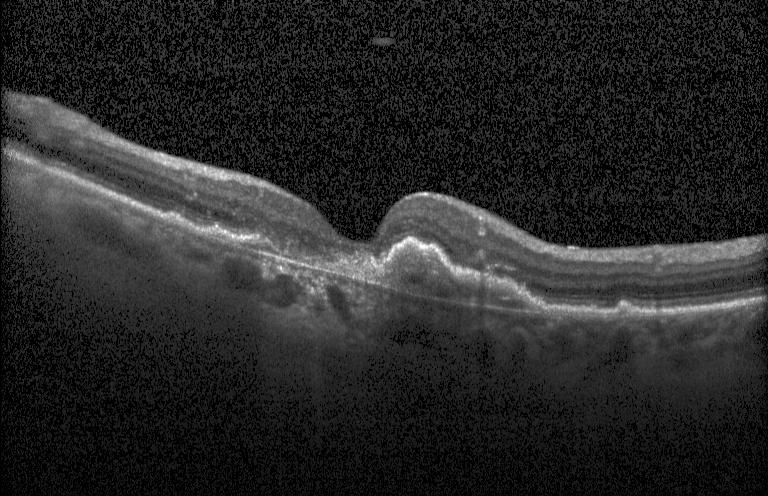
Heidelberg Spectralis. Spectral-domain OCT. Retinal OCT cross-section.
This B-scan demonstrates choroidal neovascularization (CNV).